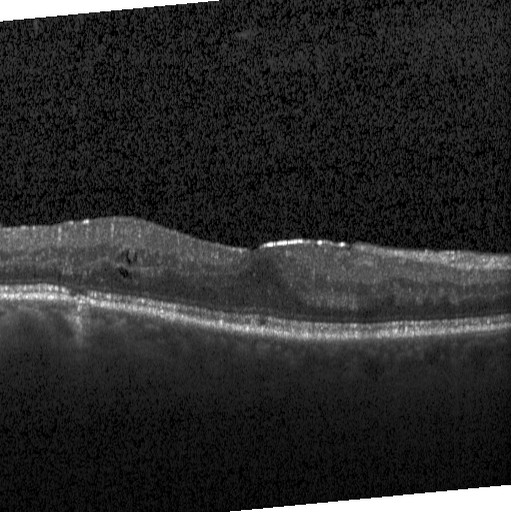 OCT finding: DME.